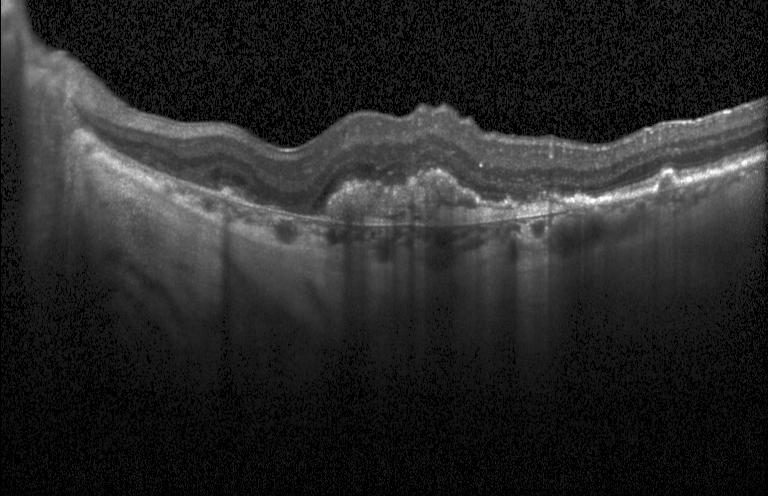
OCT B-scan; spectral-domain optical coherence tomography; macular scan. Impression: a choroidal neovascular membrane.